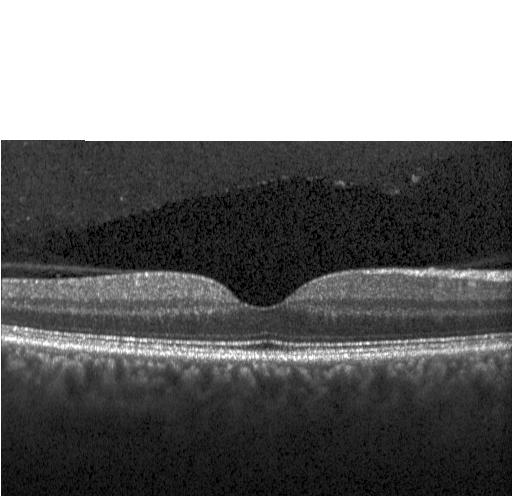
Assessment: neither CNV, DME, nor drusen.